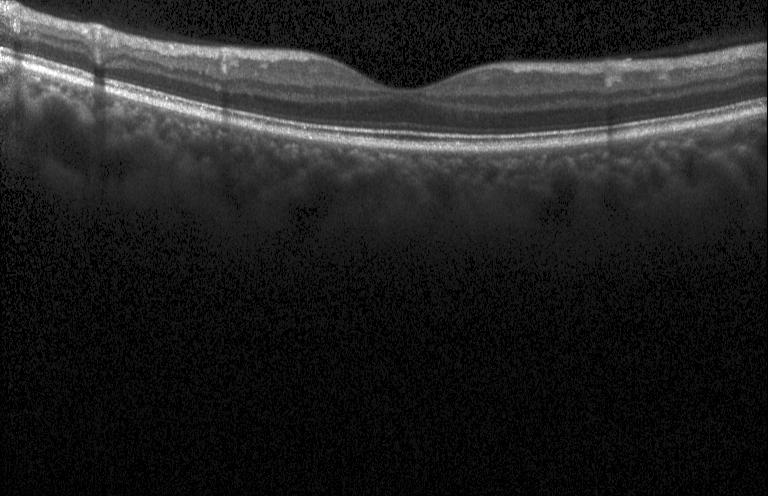 Acquired on a Heidelberg Spectralis; spectral-domain optical coherence tomography; optical coherence tomography B-scan.
Macular OCT: neither choroidal neovascularization, diabetic macular edema, nor drusen.